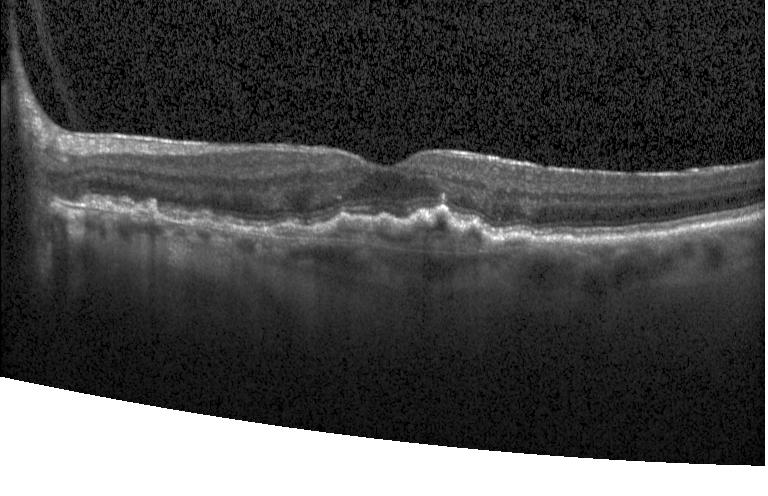
Macular OCT demonstrating a choroidal neovascular membrane.